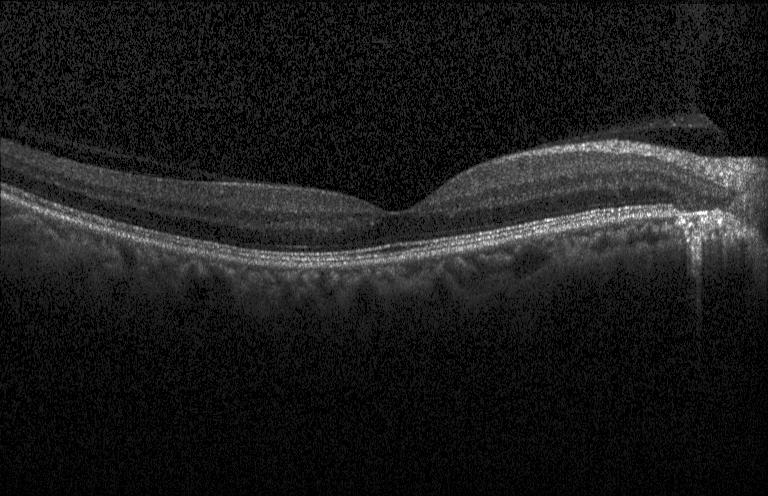 Spectral-domain optical coherence tomography, Heidelberg Spectralis, optical coherence tomography B-scan, macular scan
This B-scan demonstrates no choroidal neovascularization, no diabetic macular edema, and no drusen.